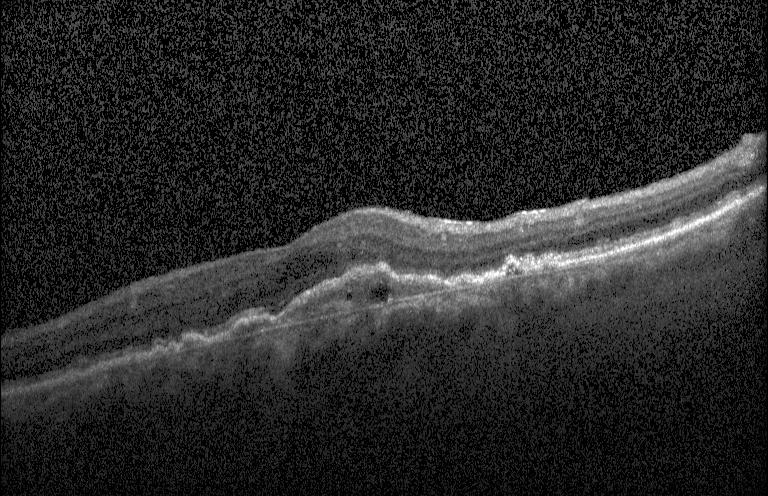
Spectral-domain optical coherence tomography; OCT line scan; horizontal scan through the fovea. Macular OCT: choroidal neovascularization.